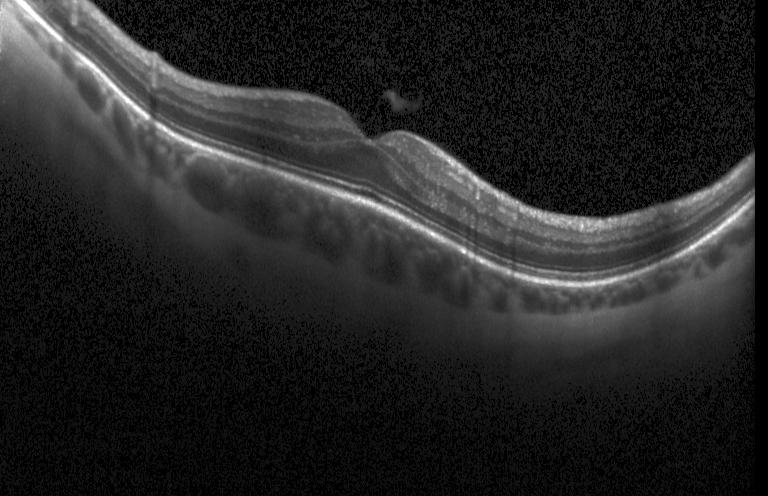 Centered on the fovea. Retinal OCT B-scan. Spectral-domain optical coherence tomography — Impression: neither choroidal neovascularization, diabetic macular edema, nor drusen.